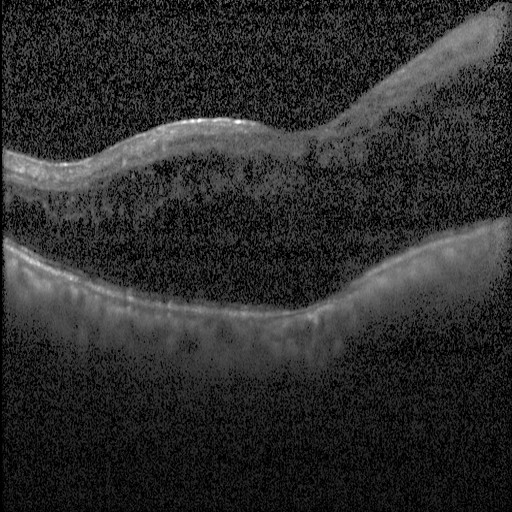

Optical coherence tomography B-scan. Macular scan — Diagnosis: DME.